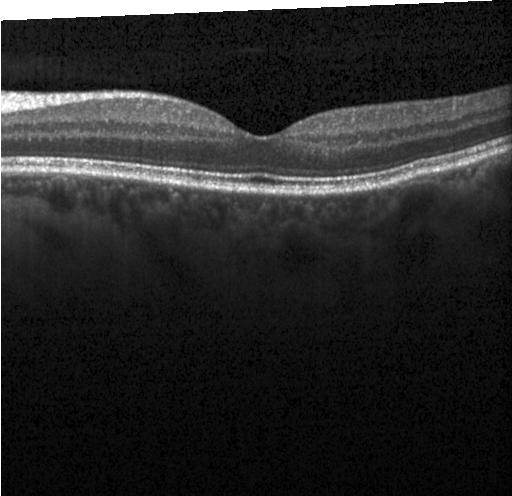 OCT line scan.
This B-scan demonstrates no choroidal neovascularization, diabetic macular edema, or drusen.